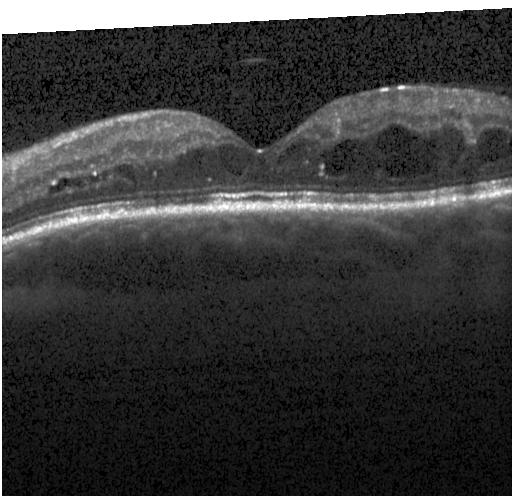

Finding: diabetic macular edema.